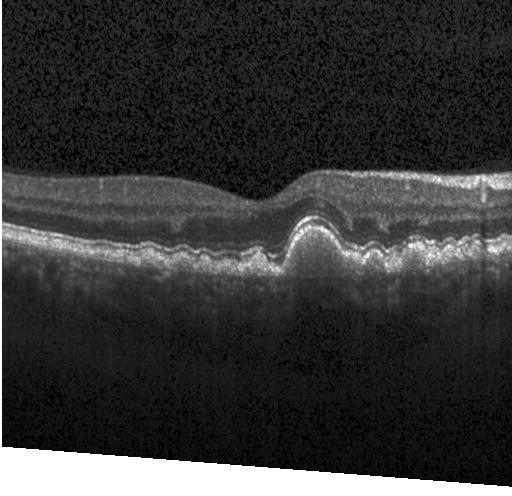
Retinal OCT B-scan · Heidelberg Spectralis · spectral-domain OCT.
Impression: sub-RPE drusenoid deposits.